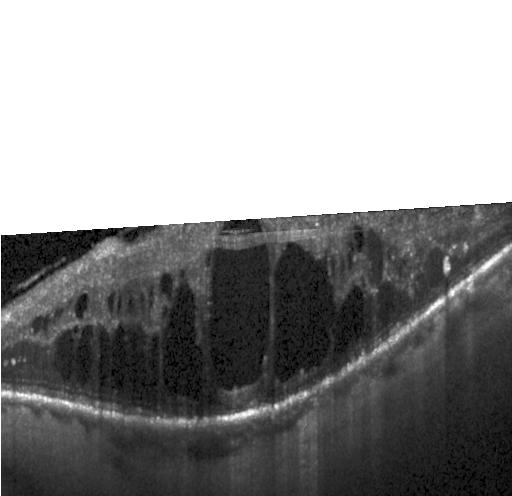
Optical coherence tomography B-scan, Heidelberg Spectralis OCT system.
This B-scan demonstrates diabetic macular edema.